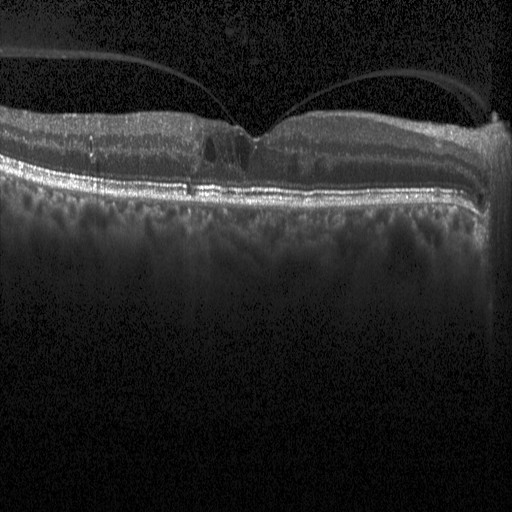 Dx: diabetic macular edema.